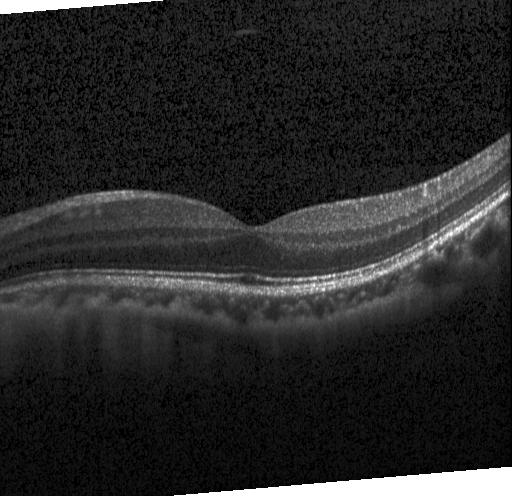

Acquired on a Heidelberg Spectralis; OCT line scan; through the macula; spectral-domain optical coherence tomography
Impression: no choroidal neovascularization, diabetic macular edema, or drusen.